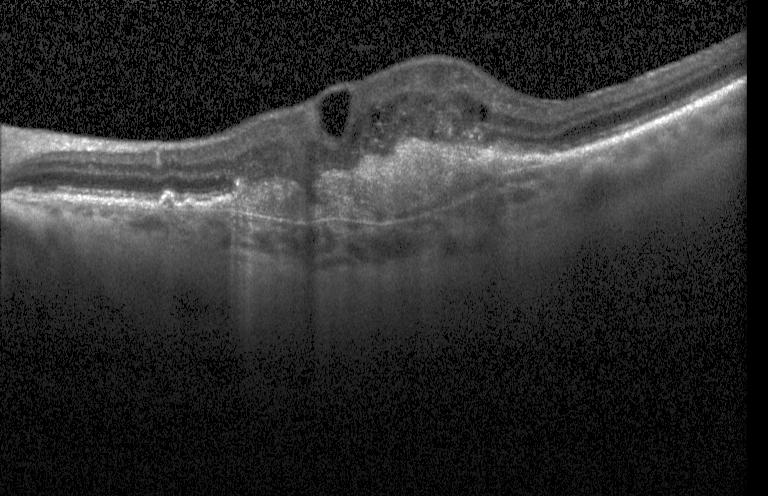 Finding: CNV.